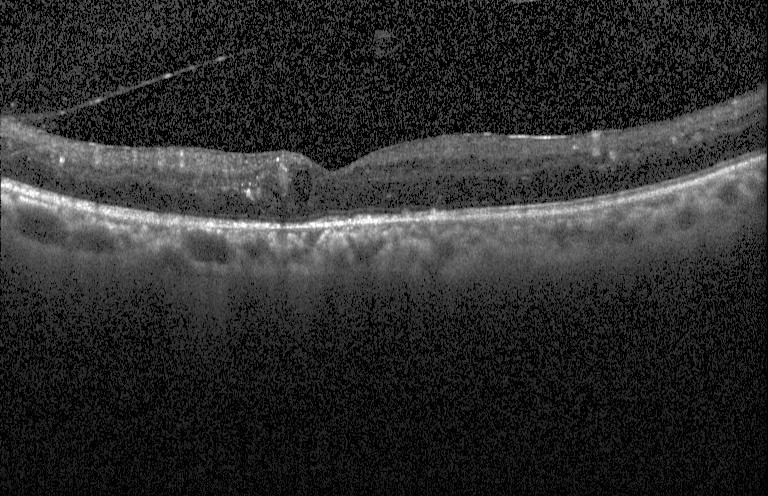 Optical coherence tomography B-scan.
Impression: DME.